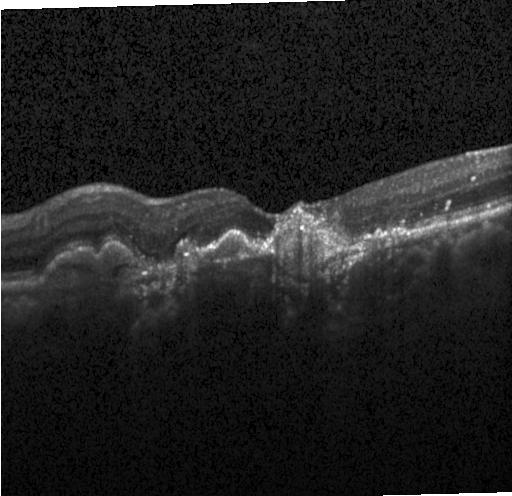

OCT finding: a choroidal neovascular membrane.